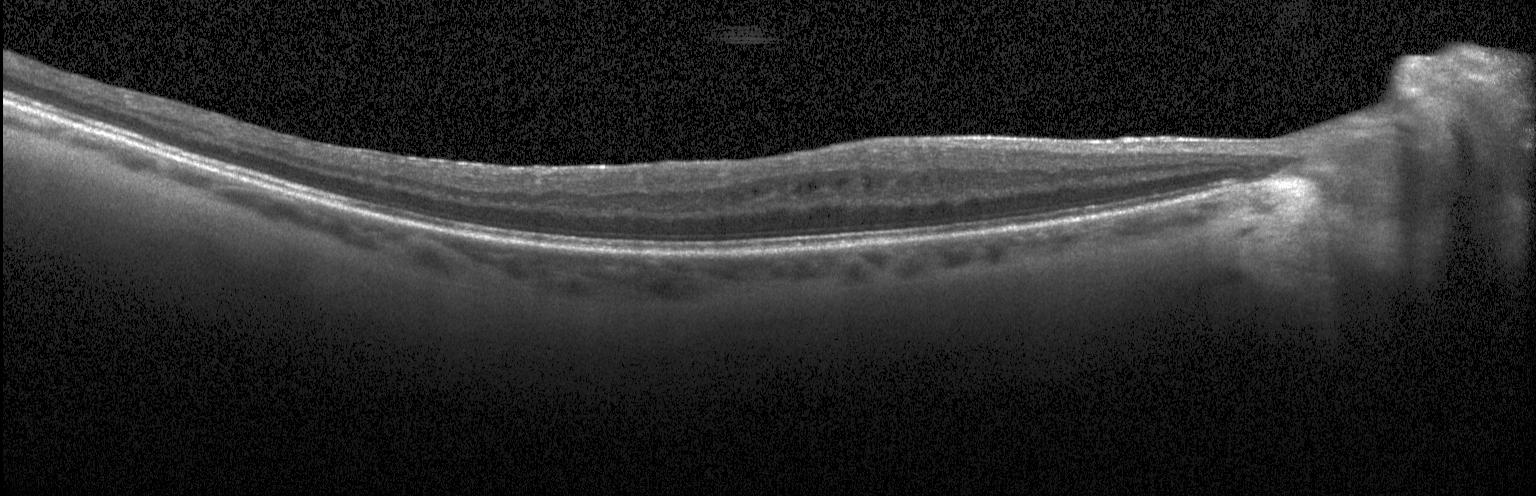

Diagnosis: DME.